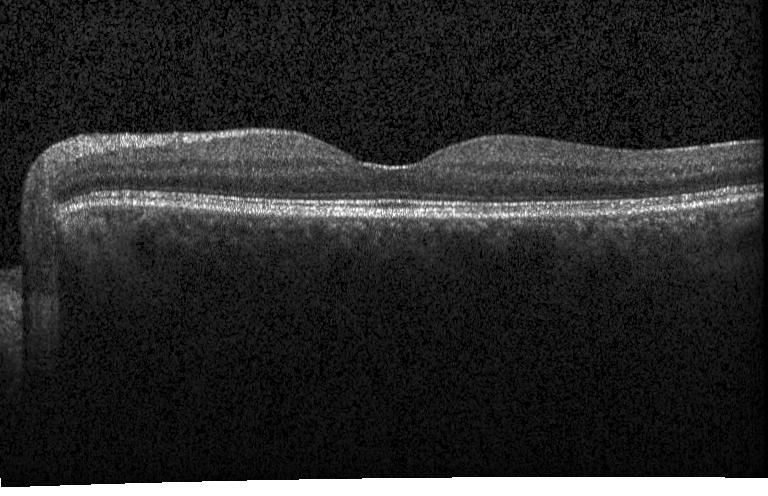 Centered on the fovea · optical coherence tomography B-scan · Heidelberg Spectralis — No evidence of CNV, DME, or drusen.